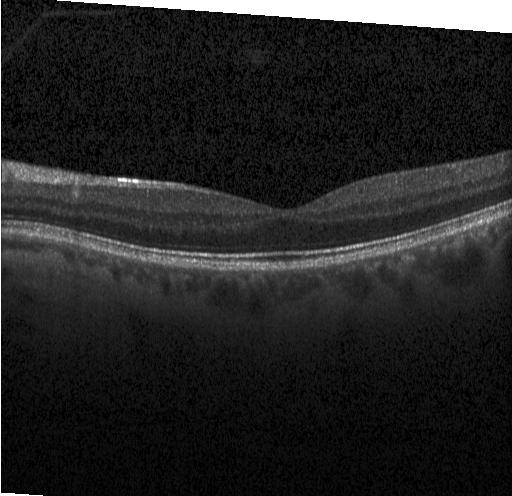 Retinal OCT cross-section, fovea-centered, spectral-domain optical coherence tomography, Heidelberg Spectralis OCT system. Macular OCT: no CNV, no DME, and no drusen.